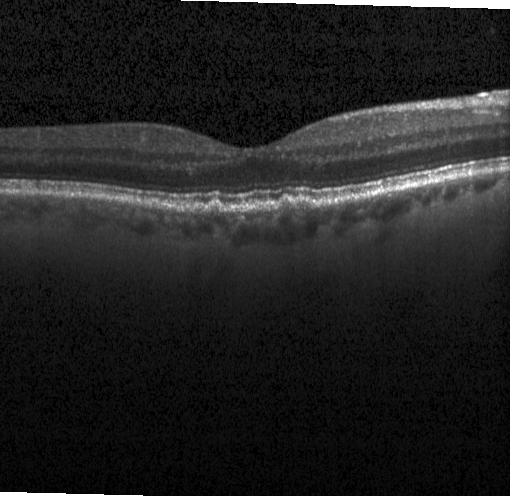

Macular OCT demonstrating sub-RPE drusenoid deposits.